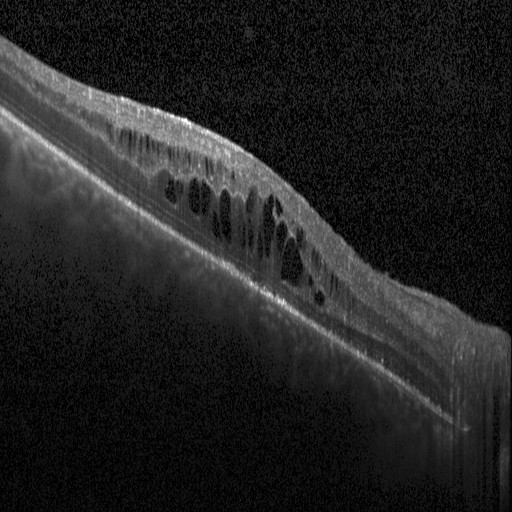 Instrument: Heidelberg Spectralis, OCT B-scan, SD-OCT — Impression: diabetic macular edema.